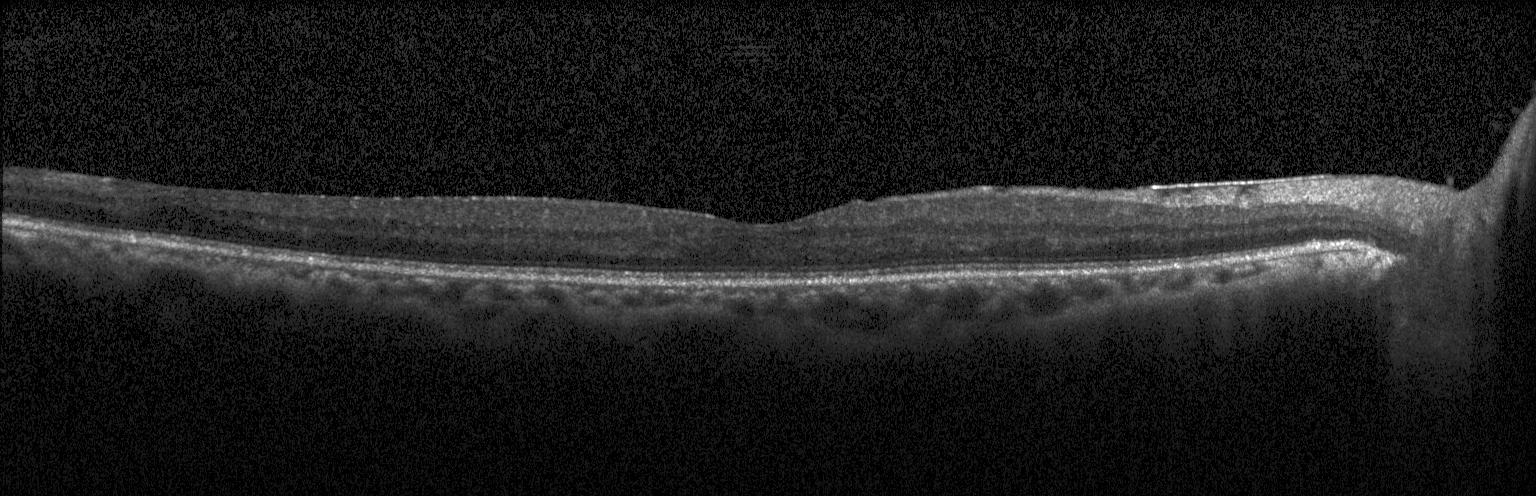 Assessment: no choroidal neovascularization, diabetic macular edema, or drusen.